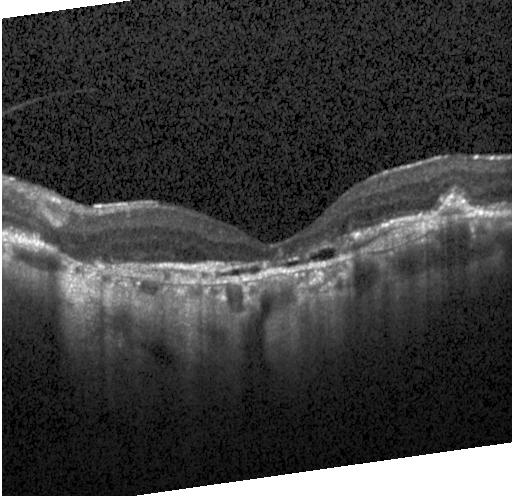

SD-OCT. Retinal OCT cross-section — The scan shows a choroidal neovascular membrane.